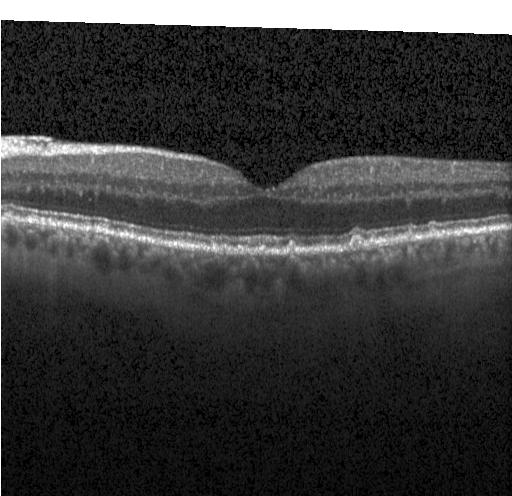 Retinal OCT cross-section showing multiple drusen.